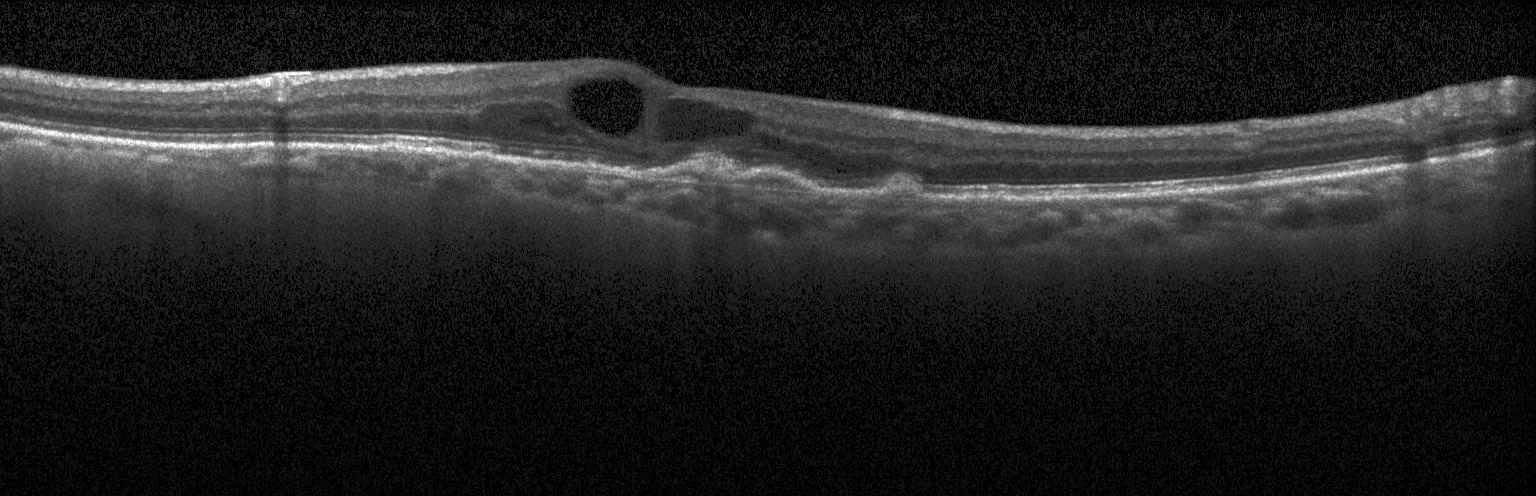
Diagnosis: a choroidal neovascular membrane.